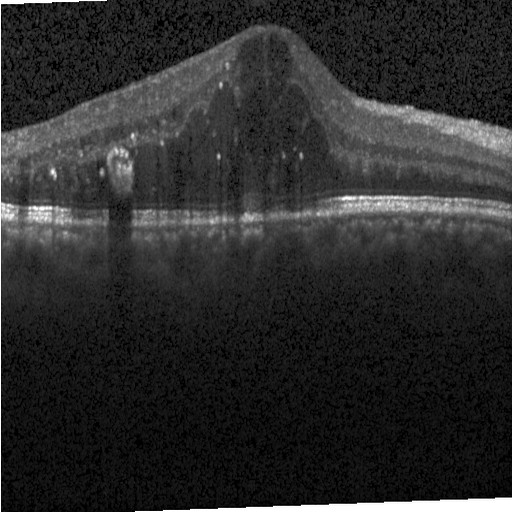

Dx: diabetic macular edema (DME).